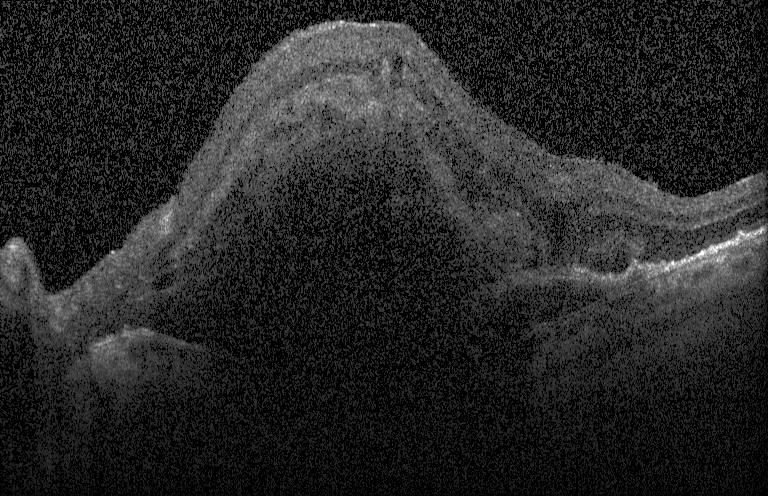
Instrument: Heidelberg Spectralis, optical coherence tomography B-scan.
Dx: choroidal neovascularization (CNV).